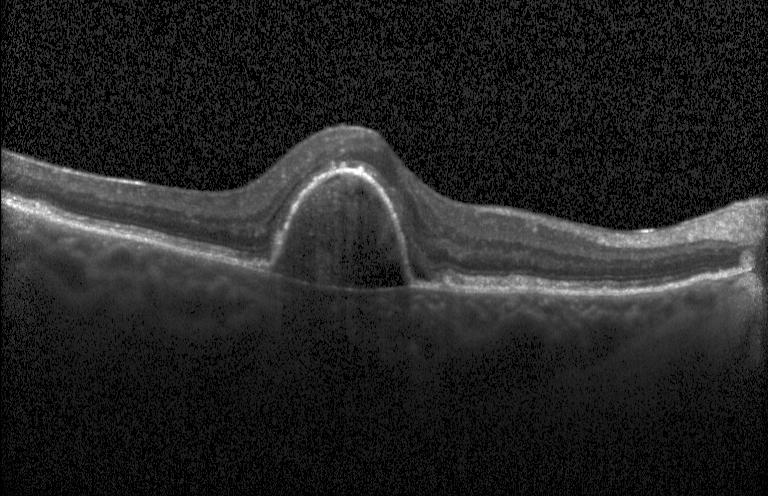
A choroidal neovascular membrane.